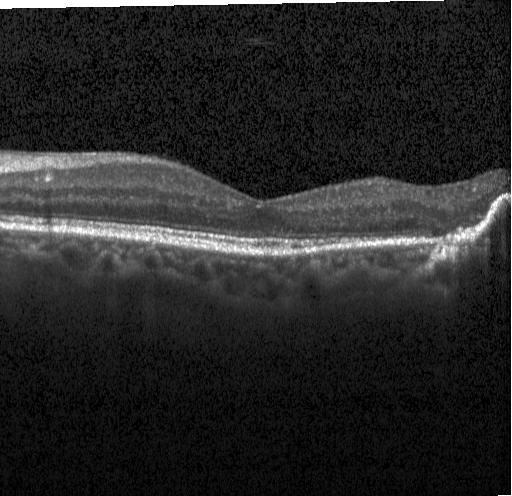 Diagnosis: a choroidal neovascular membrane.